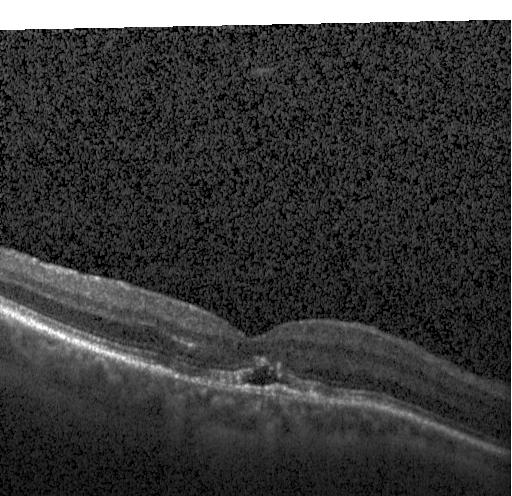
Macular OCT: choroidal neovascularization (CNV).